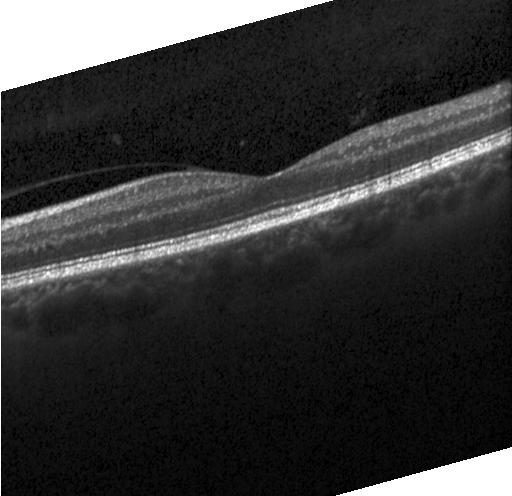
Retinal OCT B-scan. Spectral-domain optical coherence tomography
OCT finding: no choroidal neovascularization, no diabetic macular edema, and no drusen.